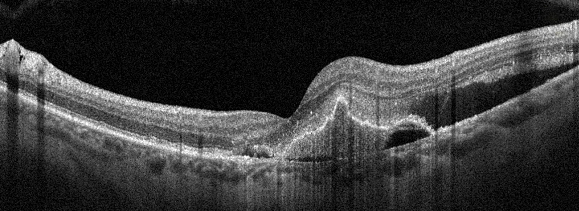 Retinal OCT B-scan. Oculus sinister
Finding: age-related macular degeneration (AMD).